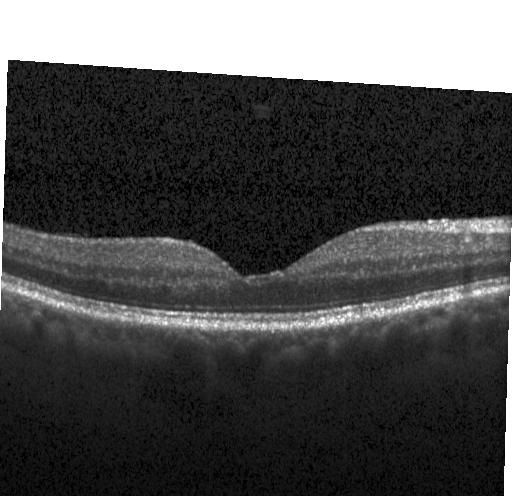

Optical coherence tomography B-scan, macular scan
Diagnosis: no CNV, no DME, and no drusen.